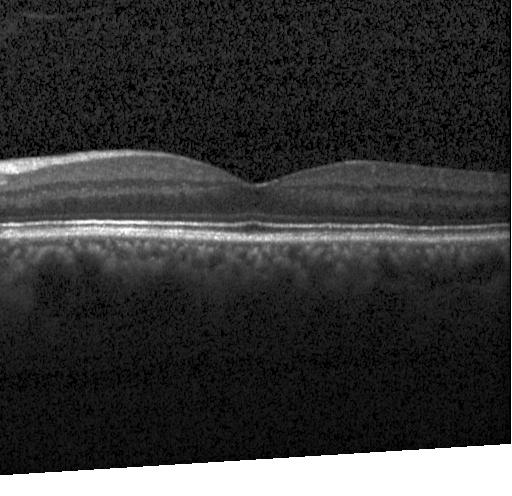
OCT B-scan; SD-OCT; Heidelberg Spectralis — Finding: no choroidal neovascularization, diabetic macular edema, or drusen.